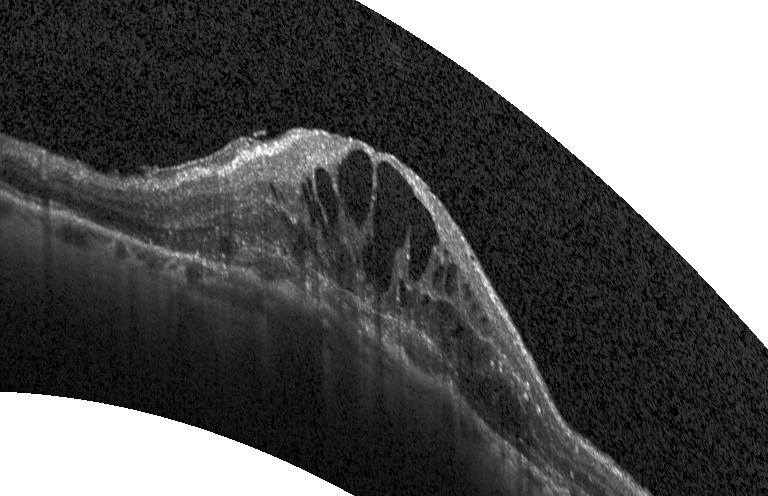 Spectral-domain OCT; optical coherence tomography scan
Finding: choroidal neovascularization.